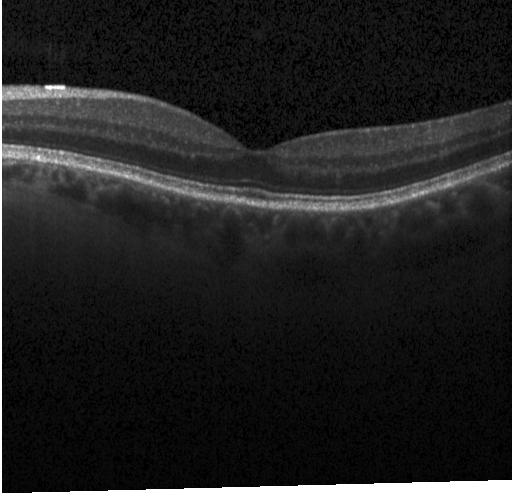

OCT line scan. Through the macula. Acquired on a Heidelberg Spectralis
This B-scan demonstrates no evidence of choroidal neovascularization, diabetic macular edema, or drusen.